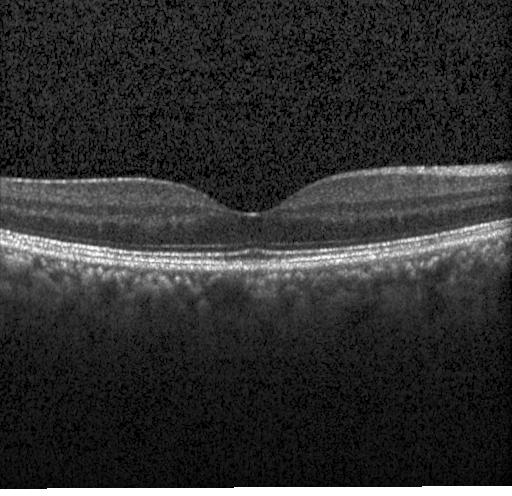 Through the macula. Instrument: Heidelberg Spectralis. Spectral-domain optical coherence tomography. Retinal OCT cross-section
The scan shows neither choroidal neovascularization, diabetic macular edema, nor drusen.